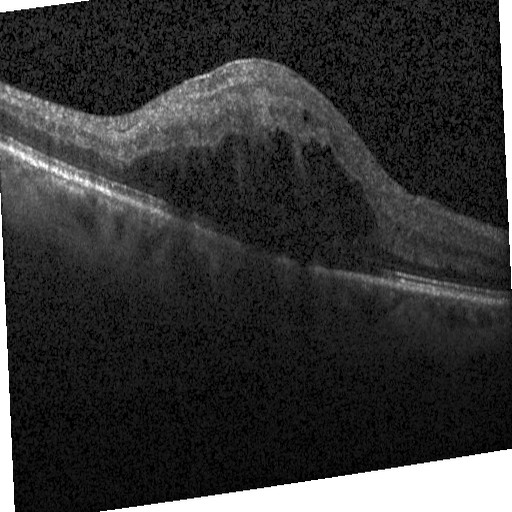
Acquired on a Heidelberg Spectralis · optical coherence tomography B-scan · spectral-domain optical coherence tomography · centered on the fovea
OCT finding: diabetic macular edema.